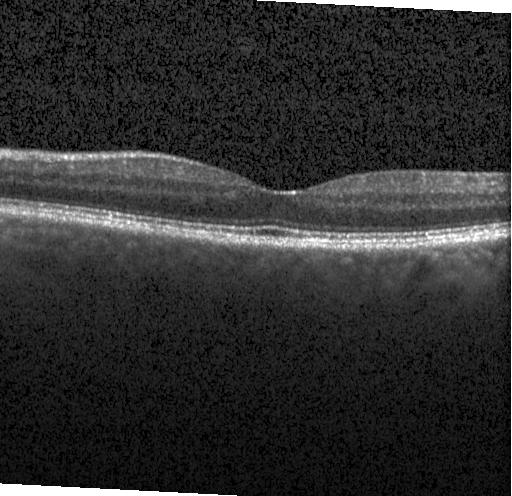
Fovea-centered; optical coherence tomography scan; SD-OCT — Assessment: no CNV, no DME, and no drusen.